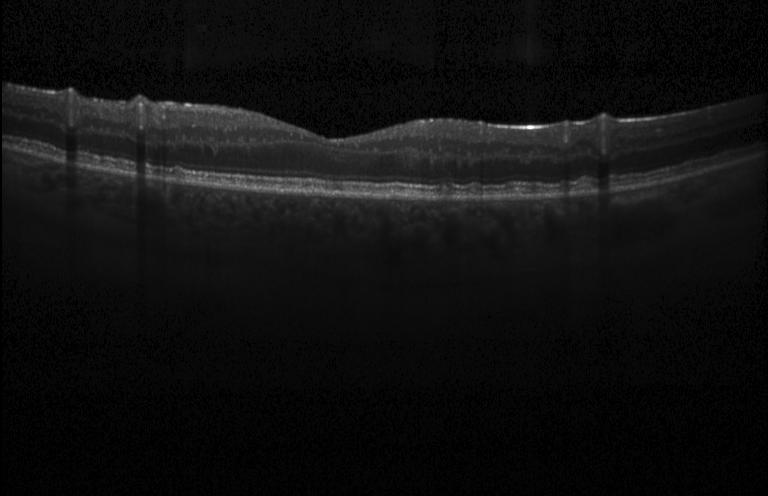 Optical coherence tomography scan.
This B-scan demonstrates multiple drusen.